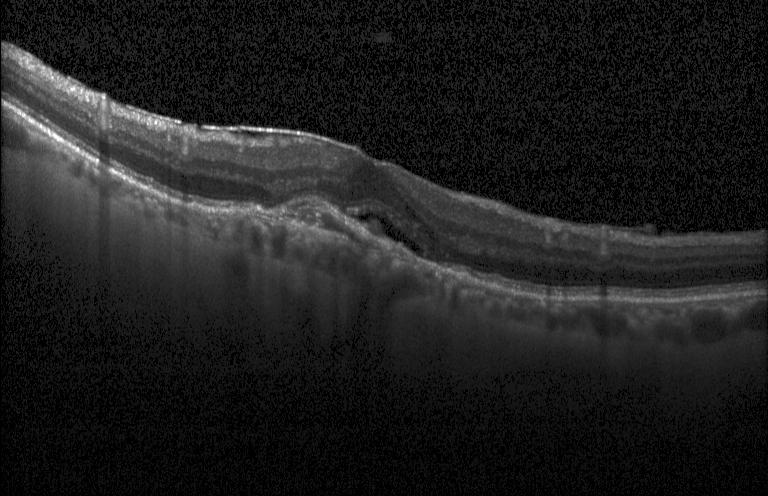
Optical coherence tomography scan; spectral-domain OCT; horizontal scan through the fovea; Heidelberg Spectralis OCT system — Diagnosis: a choroidal neovascular membrane.